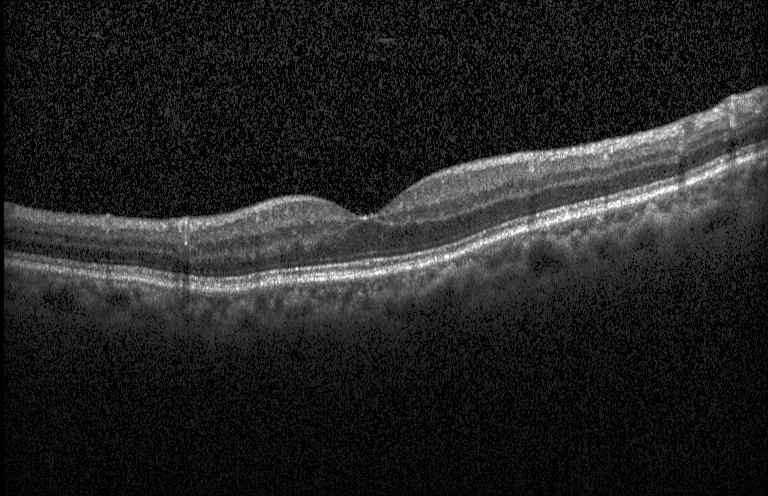

Through the macula, acquired on a Heidelberg Spectralis, SD-OCT, OCT line scan
Impression: no evidence of choroidal neovascularization, diabetic macular edema, or drusen.